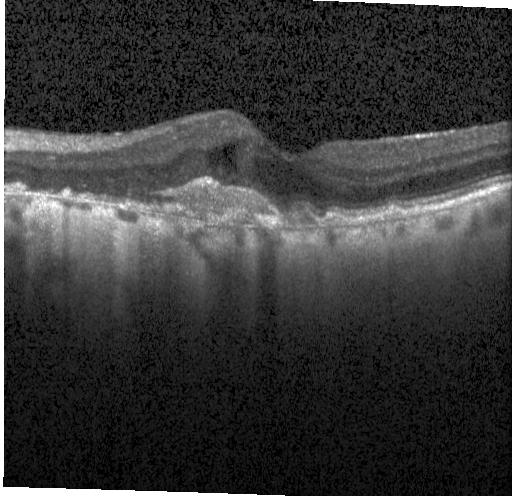
OCT B-scan showing choroidal neovascularization (CNV).